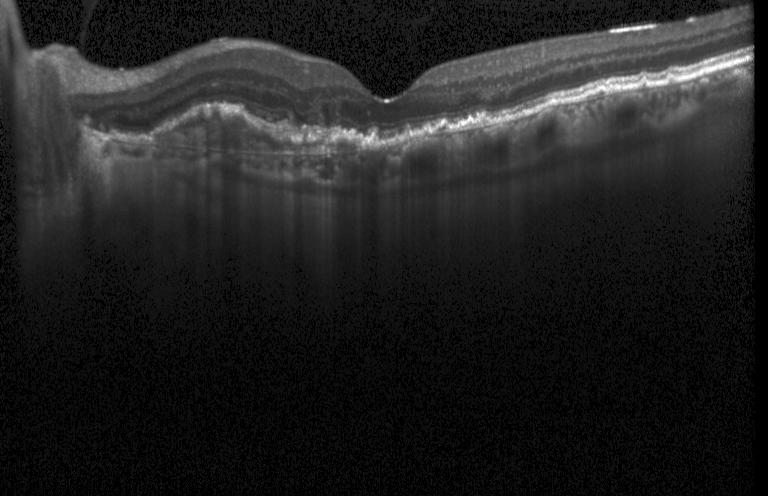
Optical coherence tomography scan — This B-scan demonstrates a choroidal neovascular membrane.